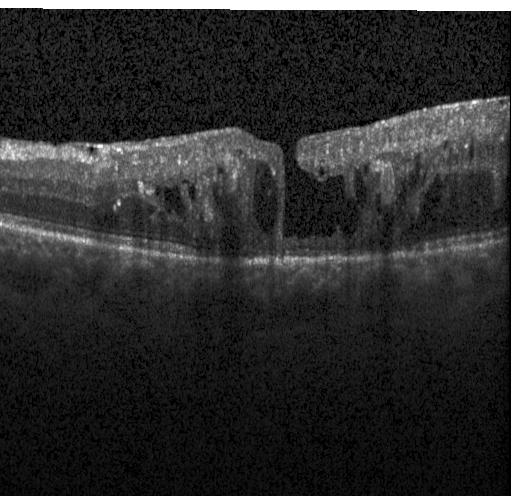 Impression: diabetic macular edema (DME).